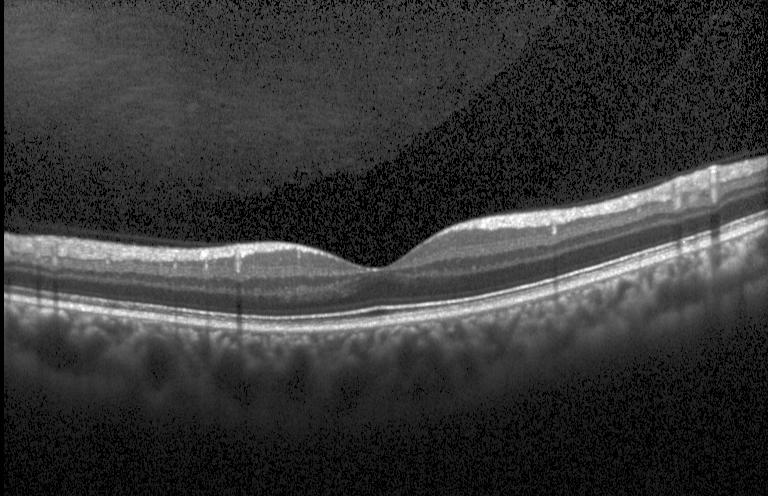
Impression: no evidence of CNV, DME, or drusen.